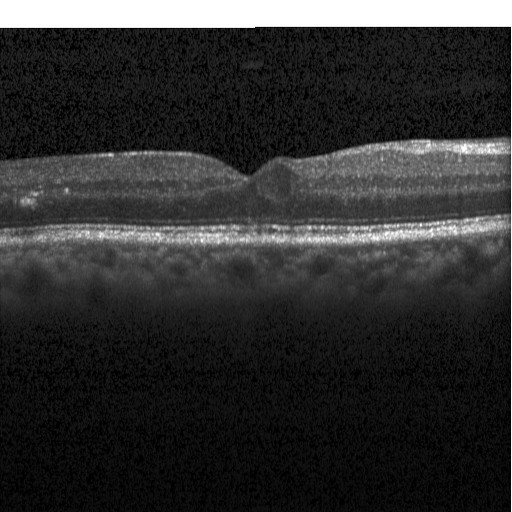
OCT finding: diabetic macular edema.